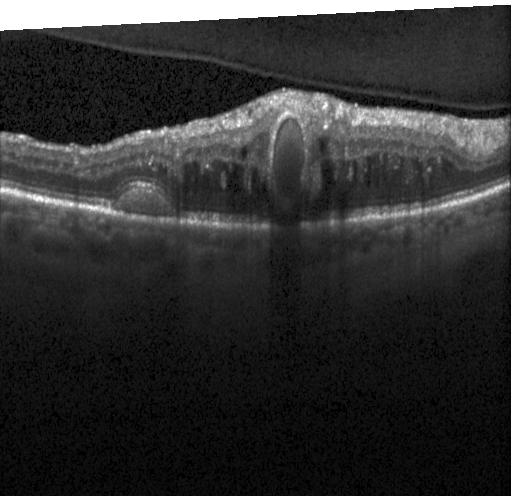
The scan shows CNV.